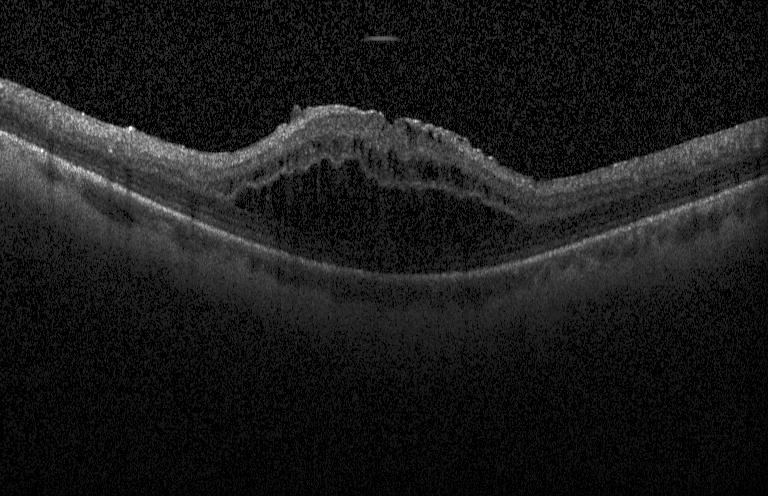
Retinal OCT B-scan.
Diagnosis: diabetic macular edema (DME).